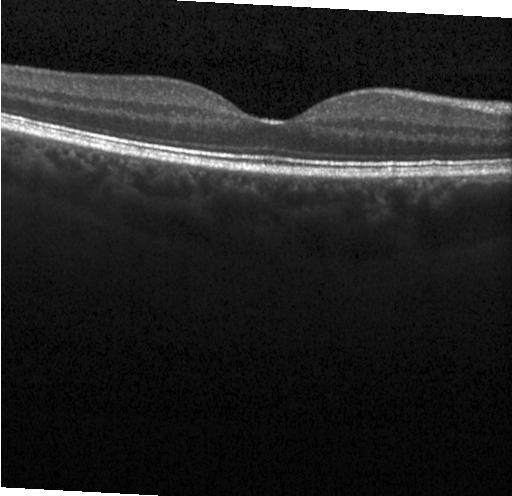
Optical coherence tomography B-scan, SD-OCT, centered on the fovea, acquired on a Heidelberg Spectralis
Finding: neither CNV, DME, nor drusen.